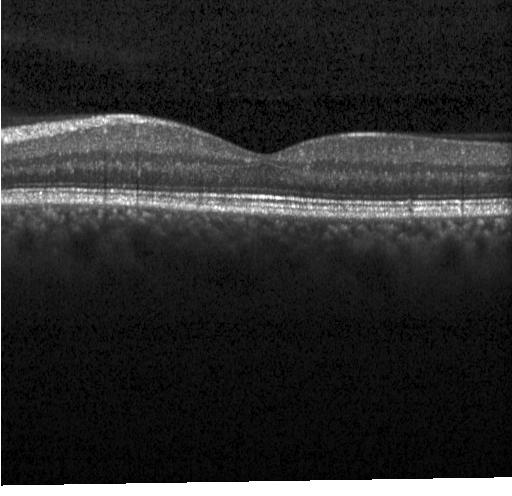

OCT B-scan.
Finding: neither choroidal neovascularization, diabetic macular edema, nor drusen.